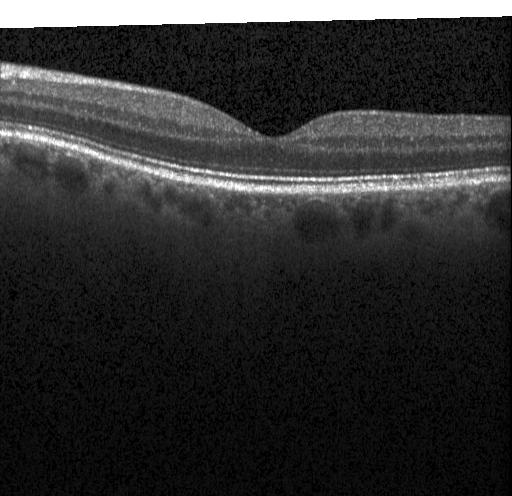
Retinal OCT B-scan; acquired on a Heidelberg Spectralis; spectral-domain OCT.
No choroidal neovascularization, diabetic macular edema, or drusen.